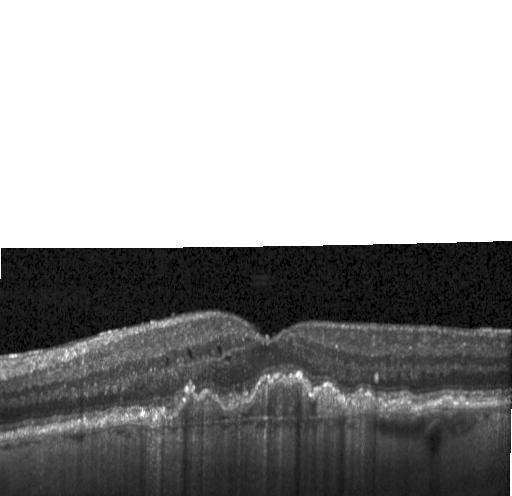

Assessment: choroidal neovascularization.